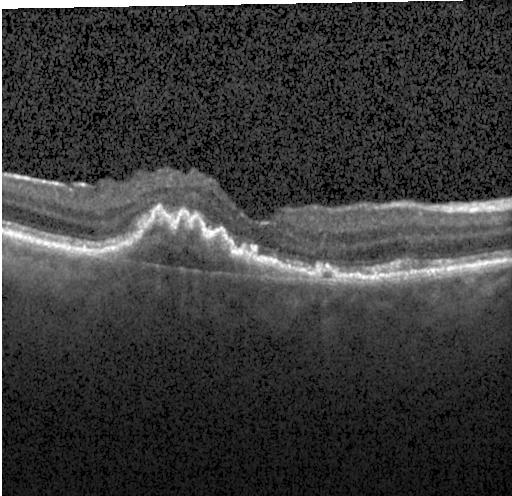

SD-OCT; OCT B-scan; fovea-centered
Diagnosis: a choroidal neovascular membrane.